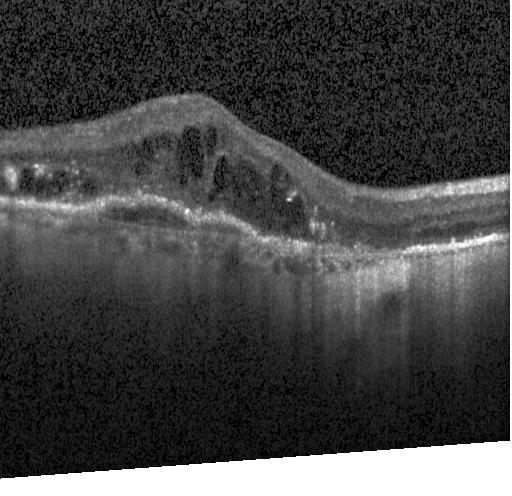

Macular scan. OCT B-scan
Impression: a choroidal neovascular membrane.